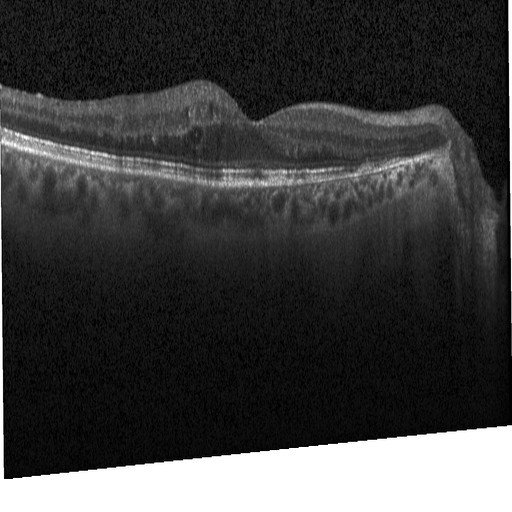

Diabetic macular edema (DME).